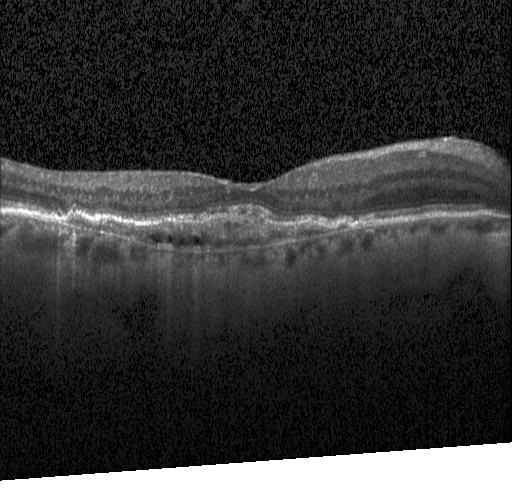
Finding: choroidal neovascularization (CNV).